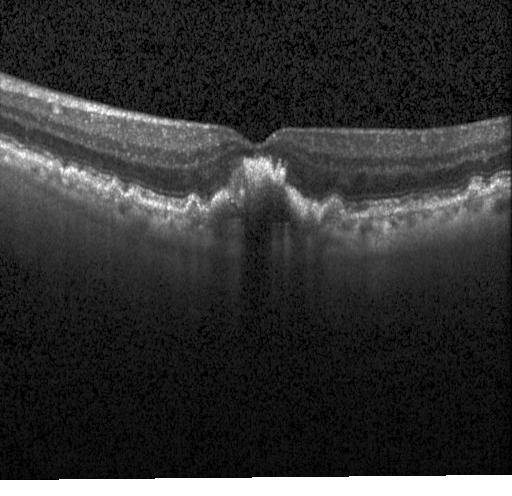
The scan shows choroidal neovascularization.